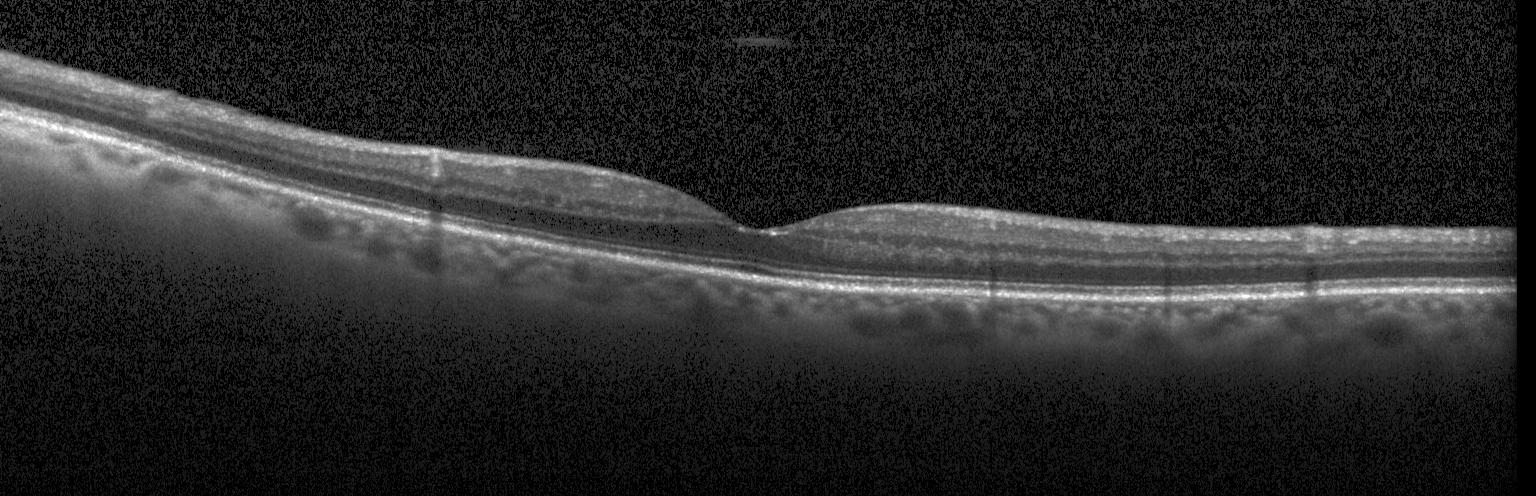

Impression: no evidence of choroidal neovascularization, diabetic macular edema, or drusen.